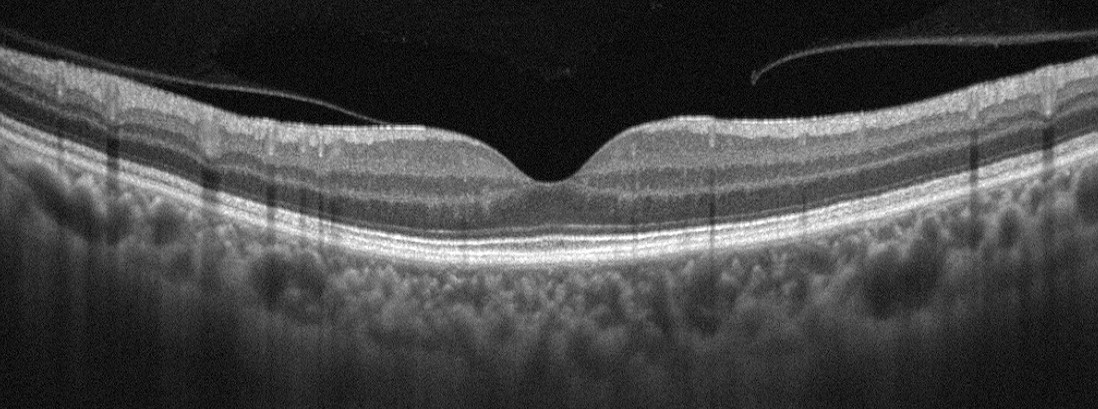 Acquired on an Optovue Avanti RTVue XR; optical coherence tomography B-scan; fovea-centered
Assessment: ERM.